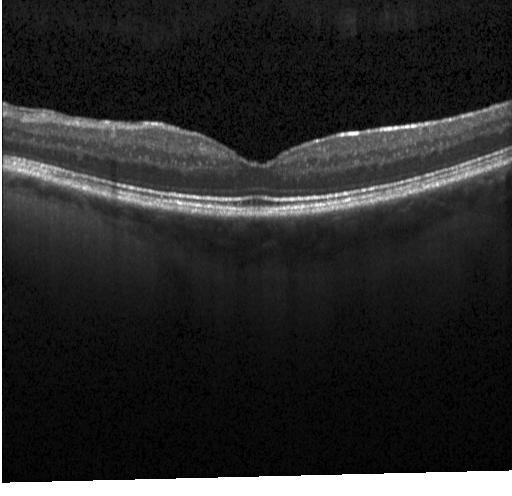
OCT scan showing no evidence of choroidal neovascularization, diabetic macular edema, or drusen.